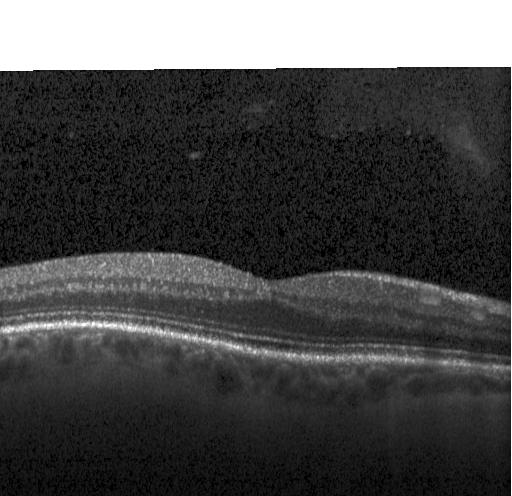 Spectral-domain OCT; macular scan; optical coherence tomography scan
Assessment: no choroidal neovascularization, no diabetic macular edema, and no drusen.